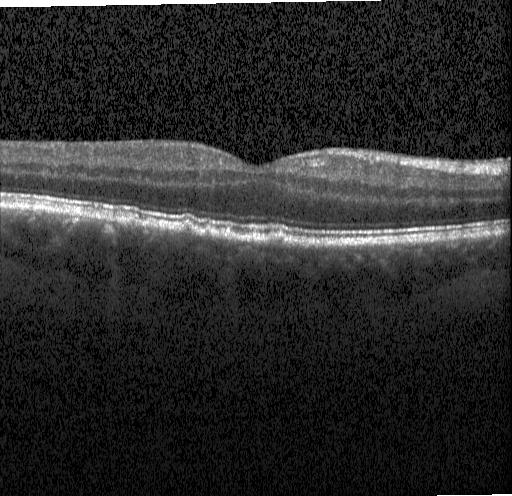

Centered on the fovea. OCT B-scan. Instrument: Heidelberg Spectralis — Sub-RPE drusenoid deposits.